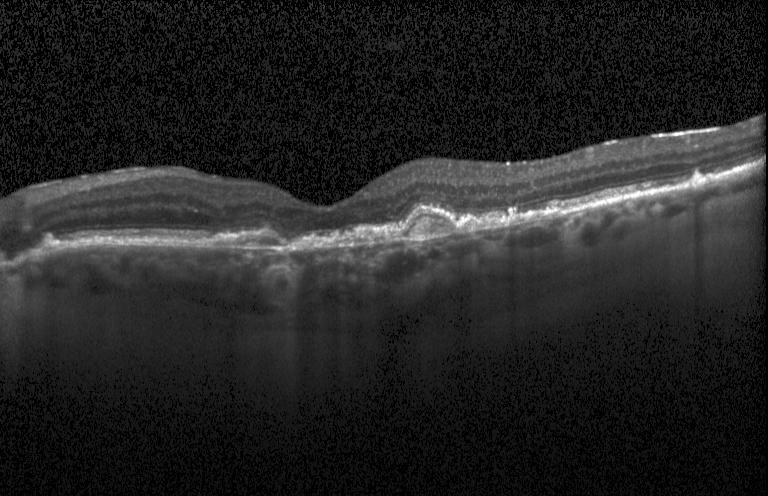
Retinal OCT cross-section. A choroidal neovascular membrane.